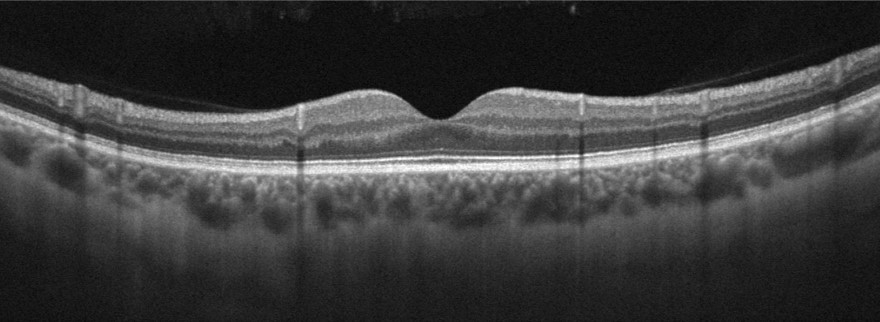 Retinal OCT B-scan · Optovue Avanti RTVue XR · fovea-centered
Impression: absence of AMD, DME, ERM, RAO, RVO, and vitreomacular interface disease.